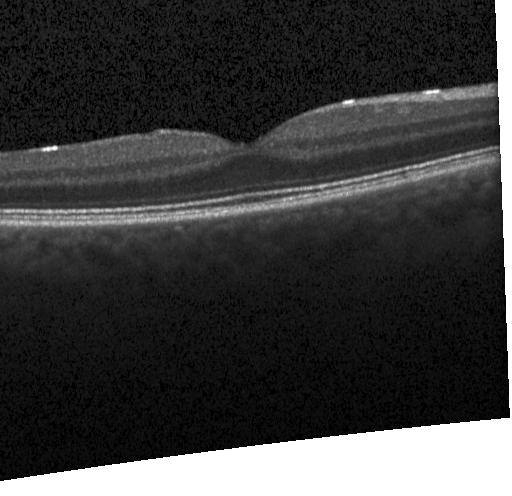
Optical coherence tomography B-scan; spectral-domain optical coherence tomography — Macular OCT: neither choroidal neovascularization, diabetic macular edema, nor drusen.